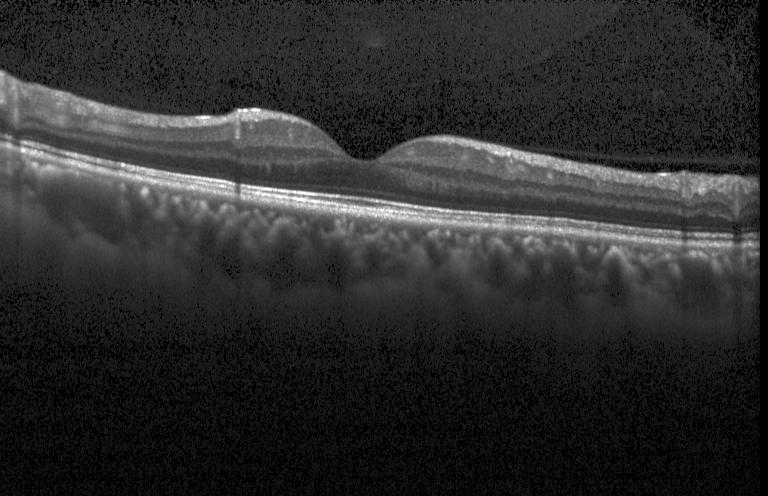

OCT B-scan, Heidelberg Spectralis OCT system — Dx: neither choroidal neovascularization, diabetic macular edema, nor drusen.